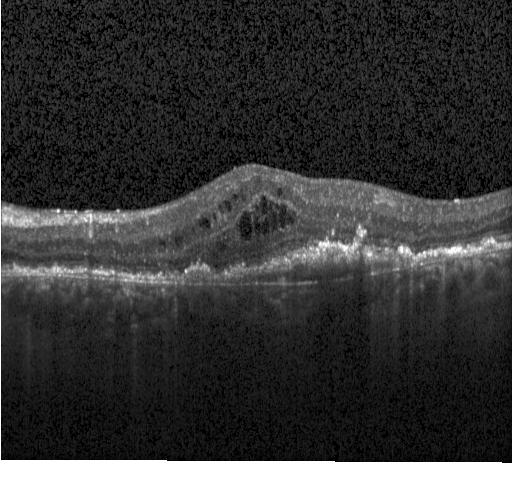

Spectral-domain OCT B-scan: a choroidal neovascular membrane.